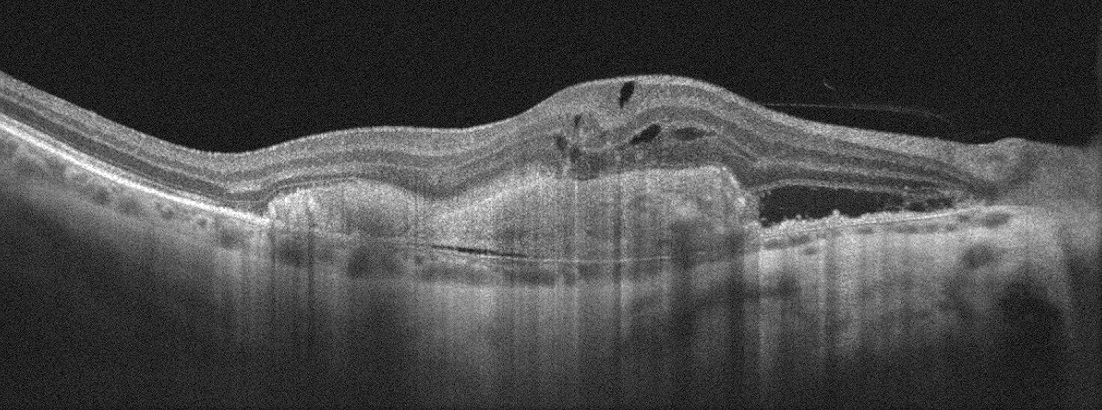

Assessment: age-related macular degeneration (AMD).